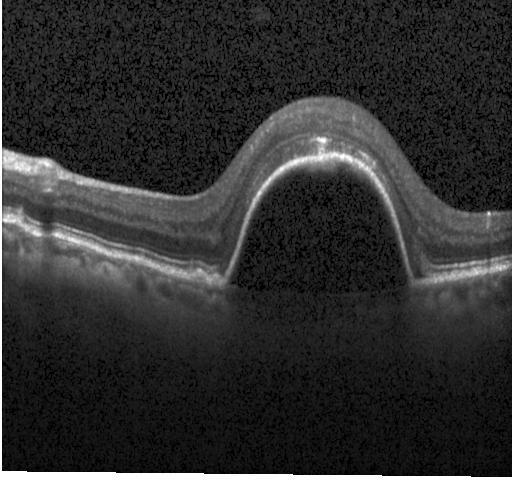 Impression: choroidal neovascularization.